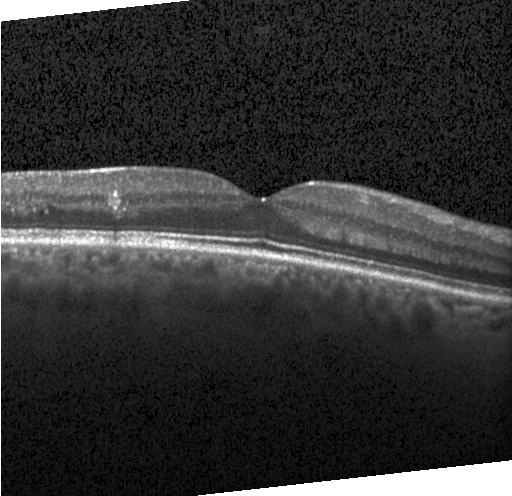
No CNV, DME, or drusen.